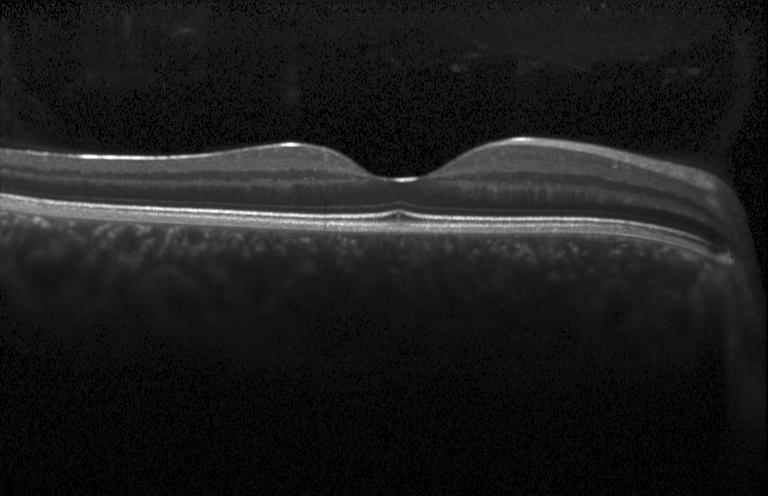 Finding: no choroidal neovascularization, no diabetic macular edema, and no drusen.